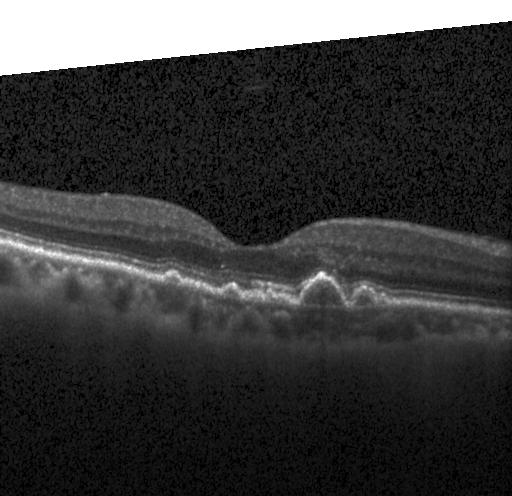 Impression: sub-RPE drusenoid deposits.